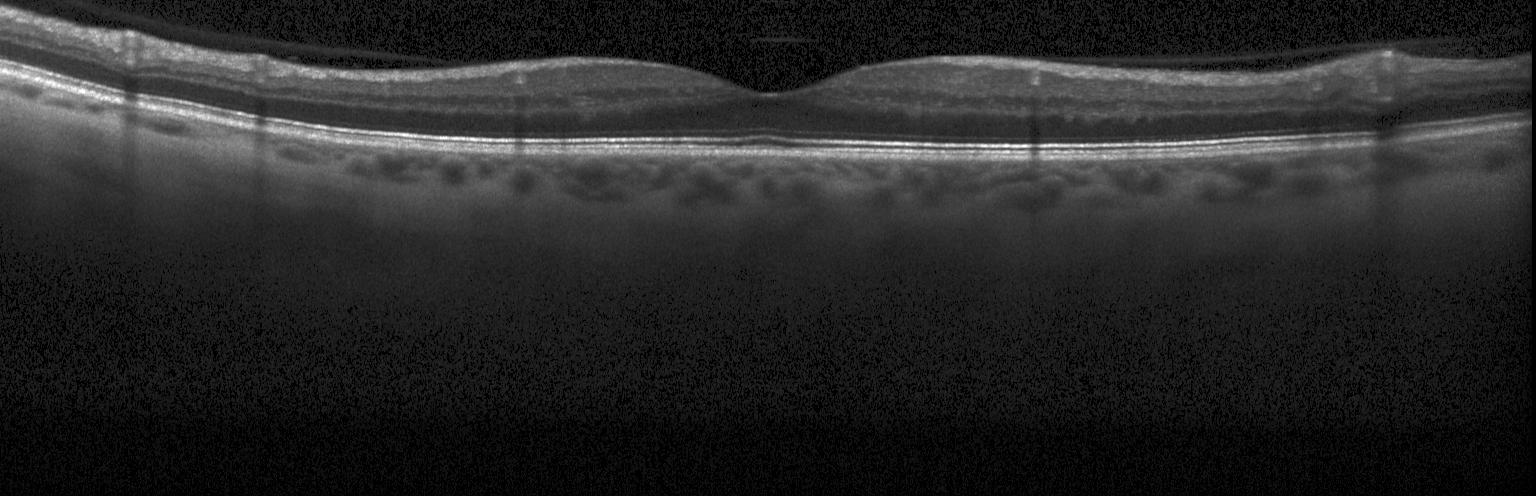 Macular scan; SD-OCT; OCT B-scan
Impression: no choroidal neovascularization, diabetic macular edema, or drusen.